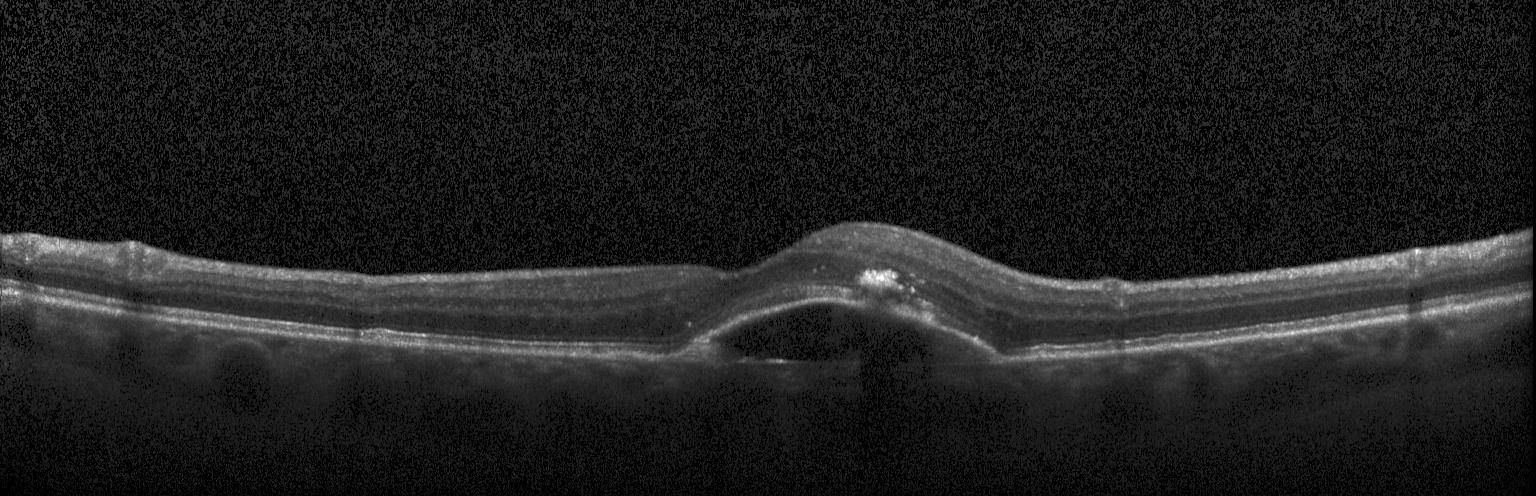

Impression: choroidal neovascularization (CNV).